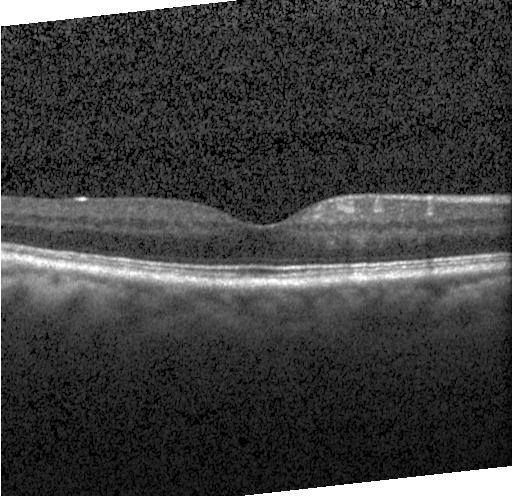

Centered on the fovea · optical coherence tomography B-scan — Impression: no evidence of CNV, DME, or drusen.